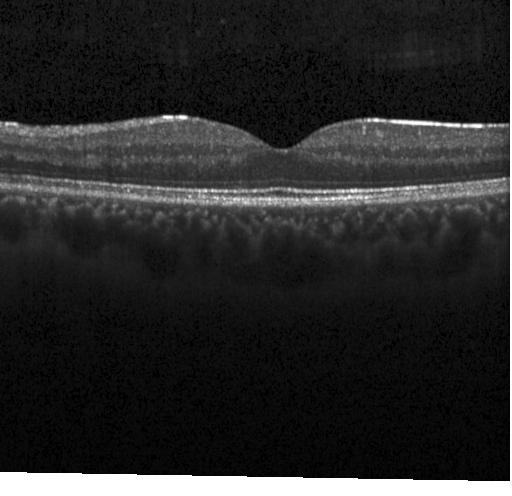 The scan shows neither choroidal neovascularization, diabetic macular edema, nor drusen.